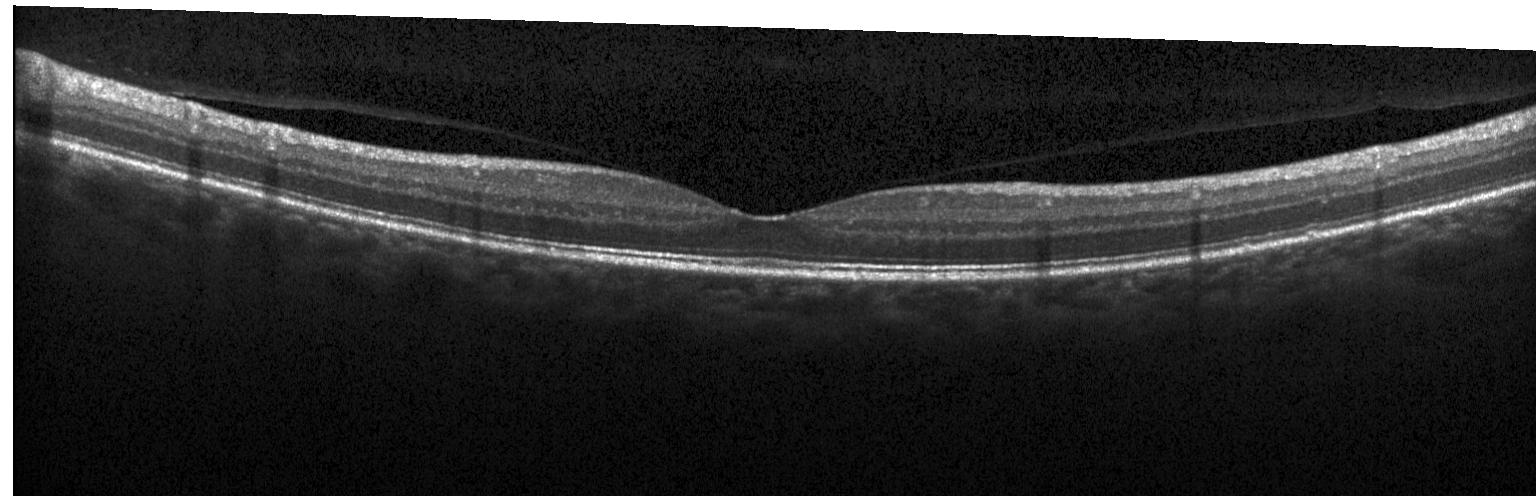 OCT line scan · horizontal scan through the fovea · spectral-domain OCT — Impression: neither choroidal neovascularization, diabetic macular edema, nor drusen.